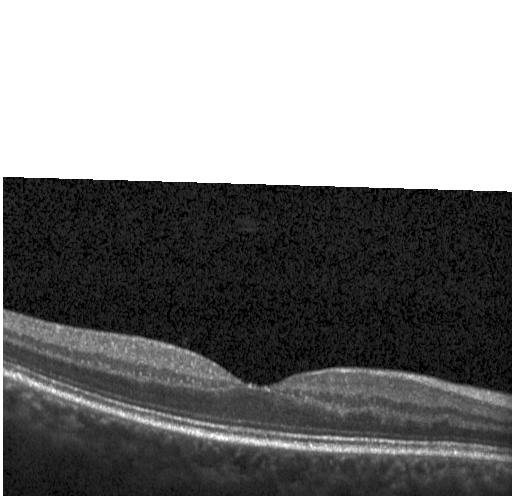

Optical coherence tomography scan · fovea-centered. Dx: no evidence of choroidal neovascularization, diabetic macular edema, or drusen.